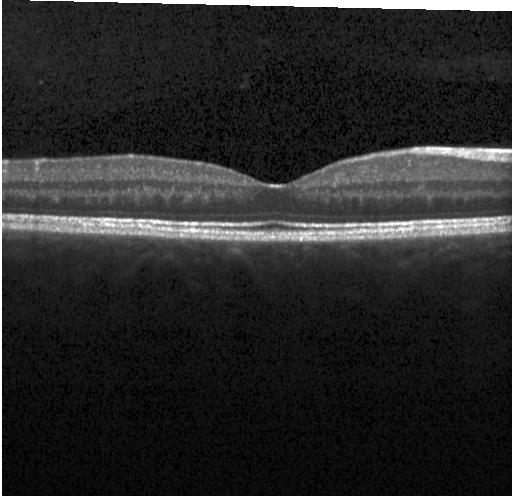

Macular scan; acquired on a Heidelberg Spectralis; spectral-domain OCT; OCT line scan — Finding: neither choroidal neovascularization, diabetic macular edema, nor drusen.